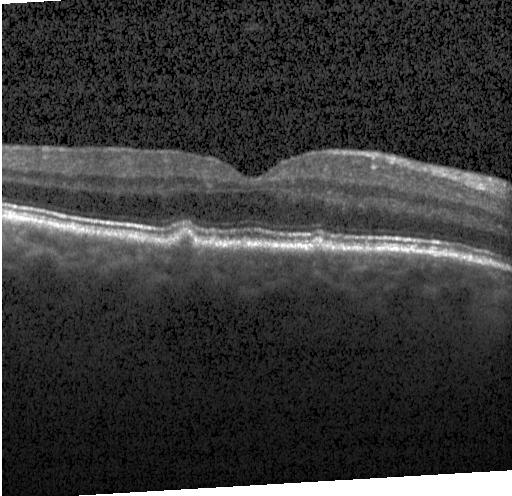 Optical coherence tomography scan, Heidelberg Spectralis OCT system — OCT finding: multiple drusen.